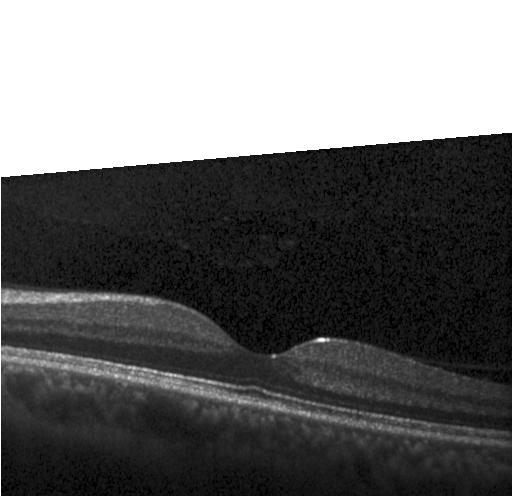
OCT B-scan showing neither CNV, DME, nor drusen.